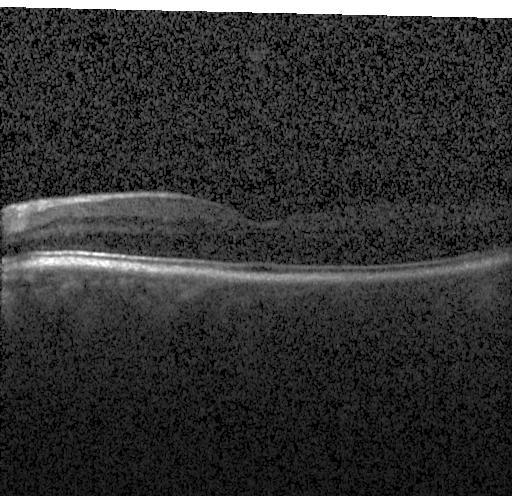

Heidelberg Spectralis OCT system; OCT line scan; macular scan; spectral-domain OCT. Diagnosis: no choroidal neovascularization, diabetic macular edema, or drusen.